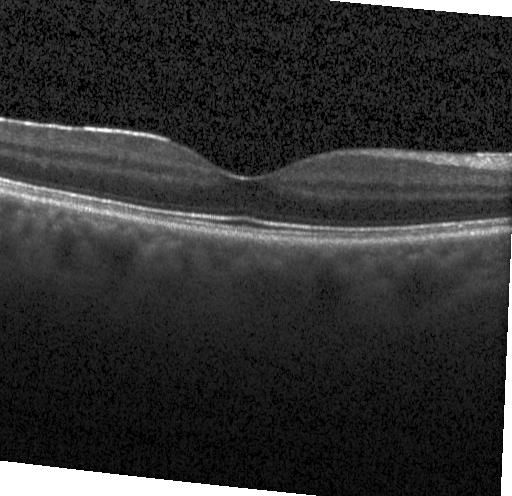
Dx: no choroidal neovascularization, diabetic macular edema, or drusen.